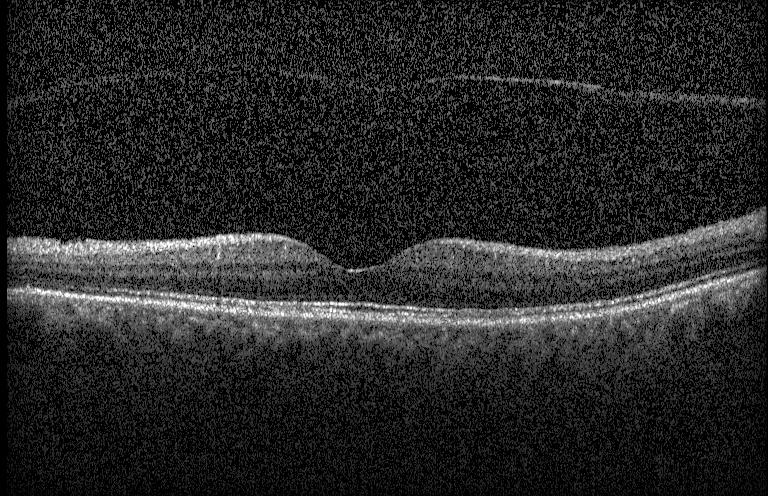

SD-OCT, instrument: Heidelberg Spectralis, through the macula, OCT B-scan — Macular OCT: neither CNV, DME, nor drusen.